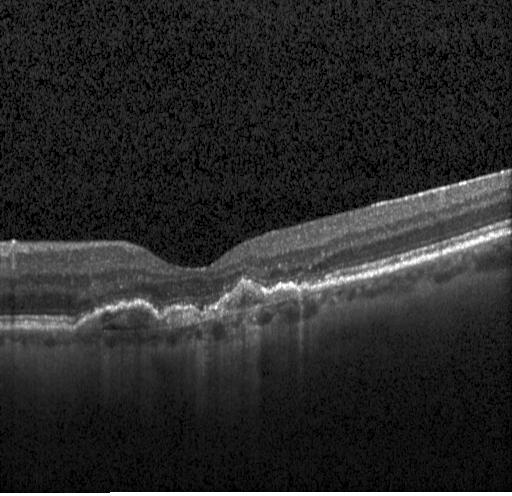

Choroidal neovascularization.